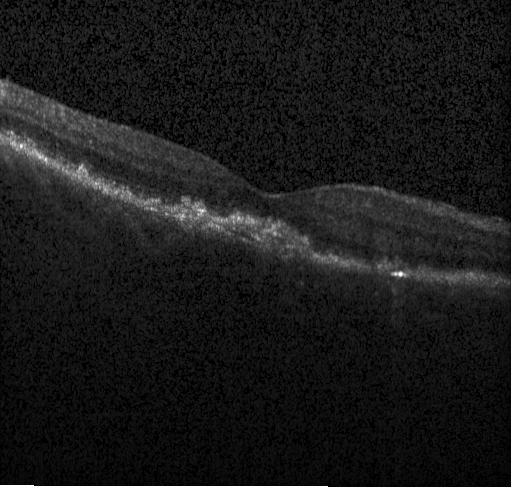 OCT B-scan · instrument: Heidelberg Spectralis — A choroidal neovascular membrane.